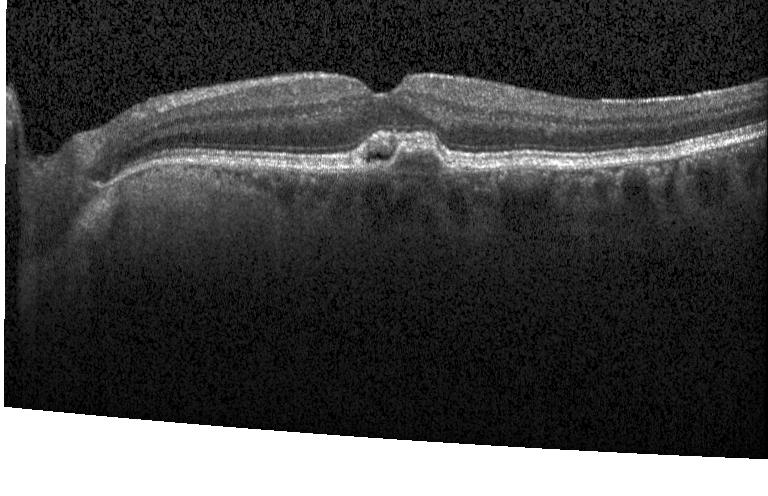
A choroidal neovascular membrane.